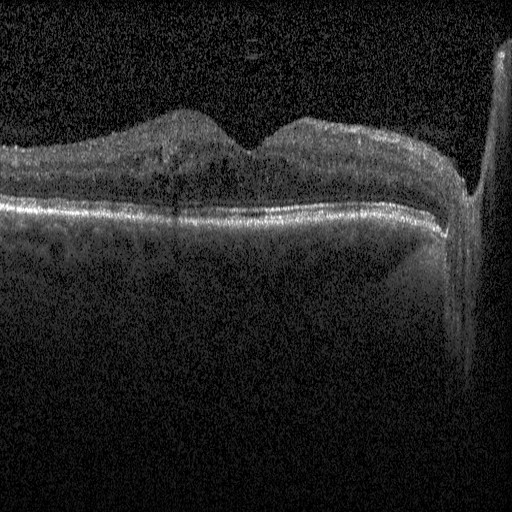
Assessment: DME.